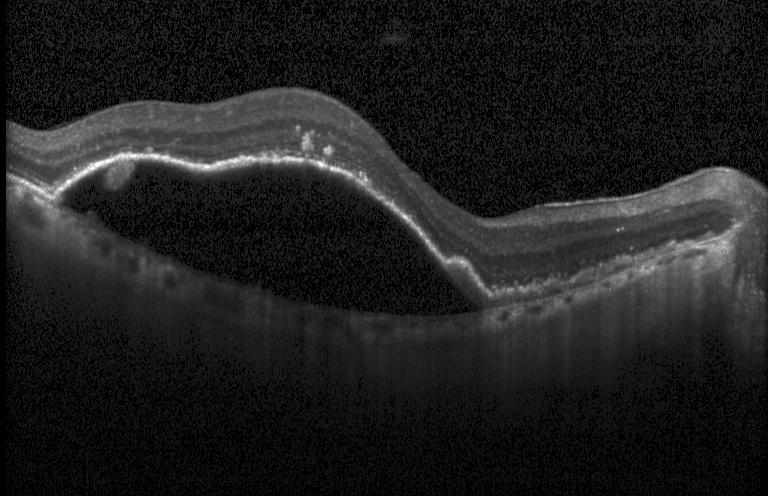 Optical coherence tomography B-scan. Dx: CNV.